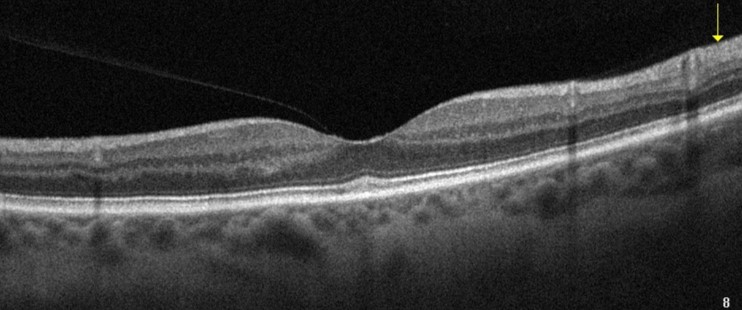
Impression: absence of AMD, DME, ERM, RAO, RVO, and vitreomacular interface disease.